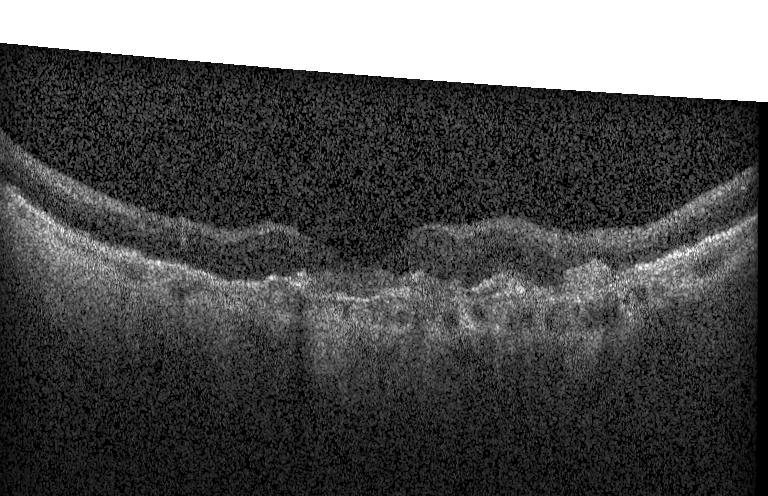

Optical coherence tomography scan.
Finding: a choroidal neovascular membrane.